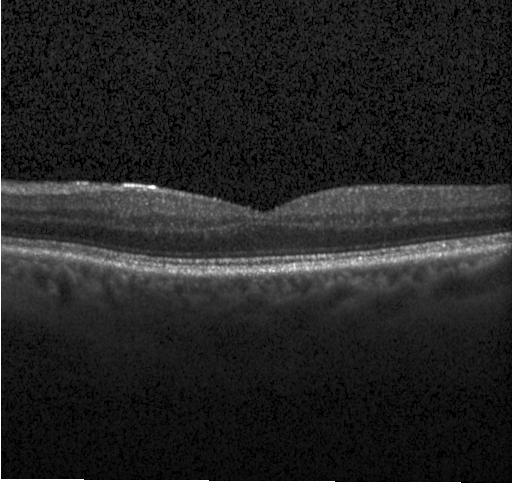 Macular scan · SD-OCT · optical coherence tomography scan. Diagnosis: no choroidal neovascularization, diabetic macular edema, or drusen.